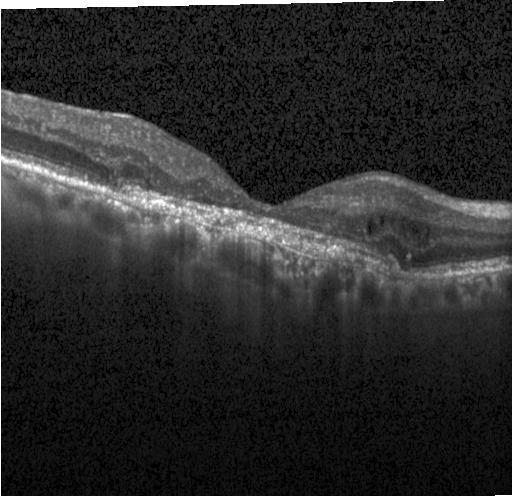
OCT B-scan showing choroidal neovascularization (CNV).